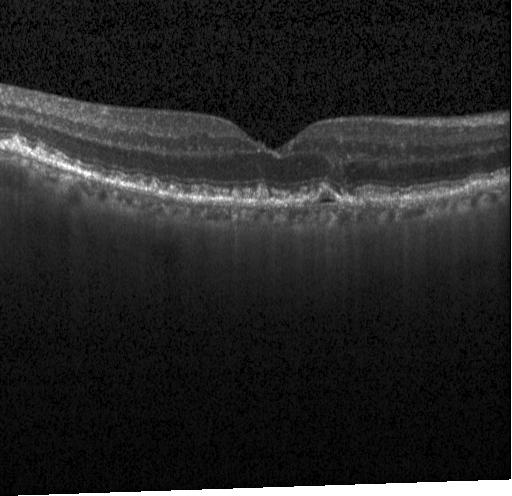
Acquired on a Heidelberg Spectralis · centered on the fovea · SD-OCT · optical coherence tomography B-scan.
Drusen.